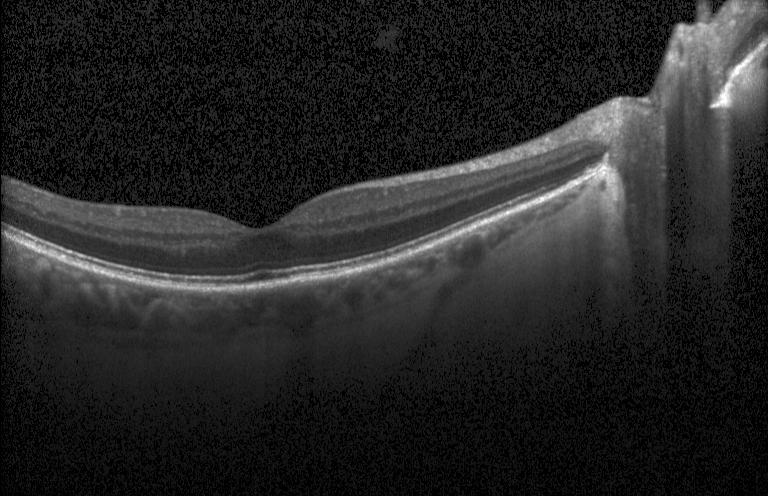 Dx: no evidence of choroidal neovascularization, diabetic macular edema, or drusen.